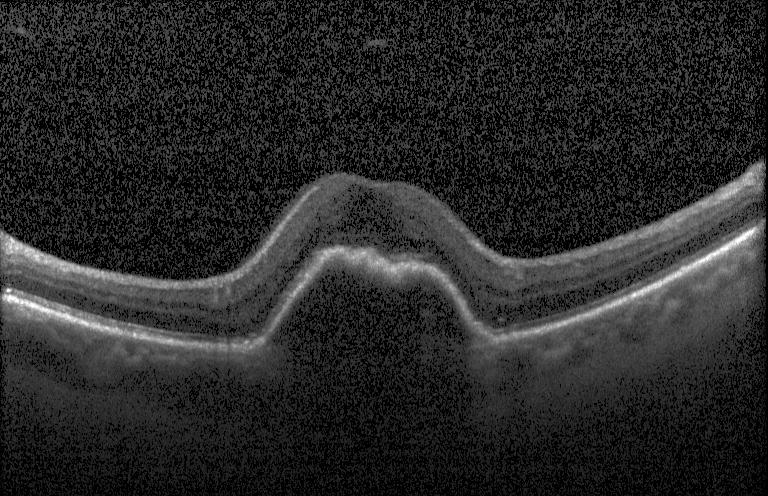

Retinal OCT cross-section, through the macula, Heidelberg Spectralis, SD-OCT.
Diagnosis: CNV.